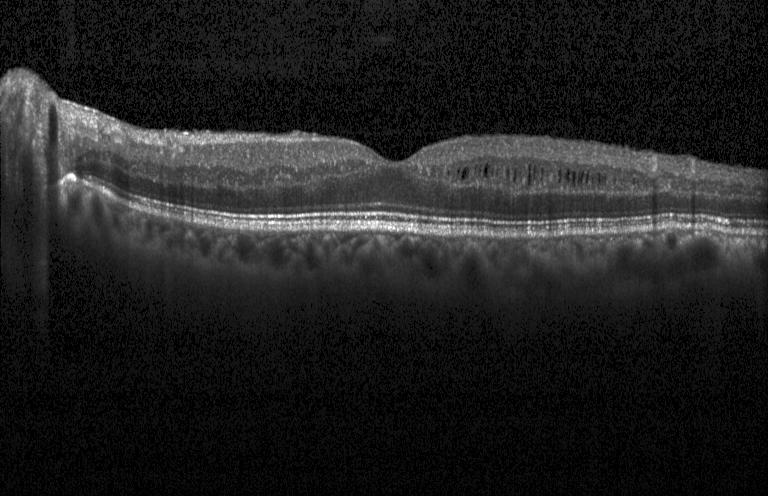 Impression: diabetic macular edema.